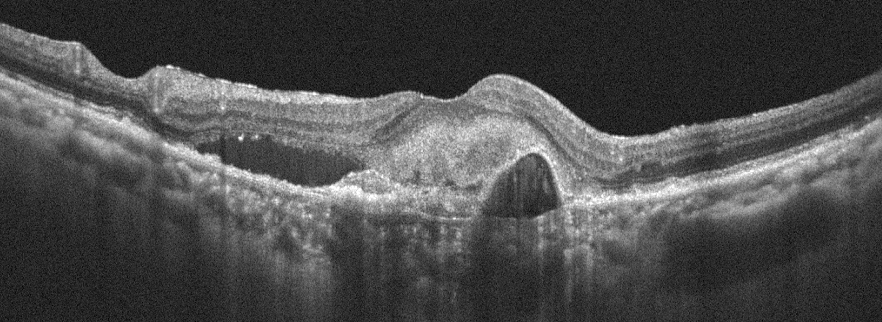 Left eye; optical coherence tomography scan. Finding: AMD.